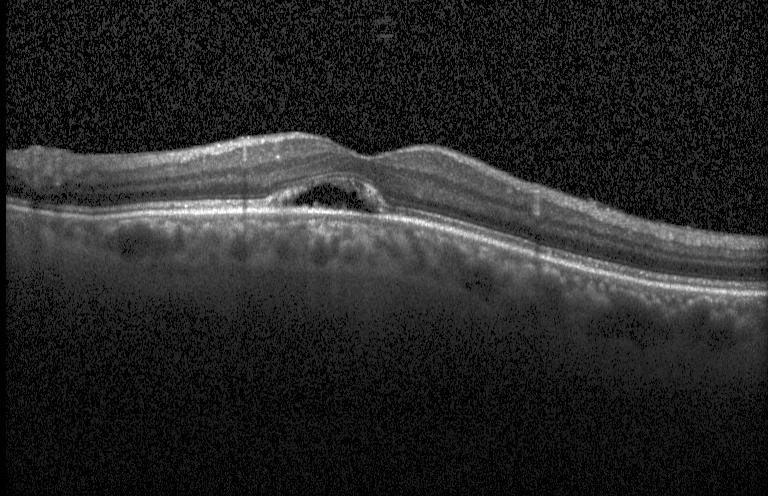
Impression: a choroidal neovascular membrane.